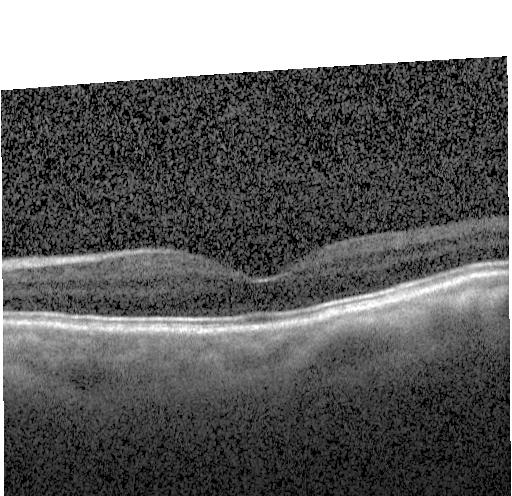
OCT finding: neither choroidal neovascularization, diabetic macular edema, nor drusen.